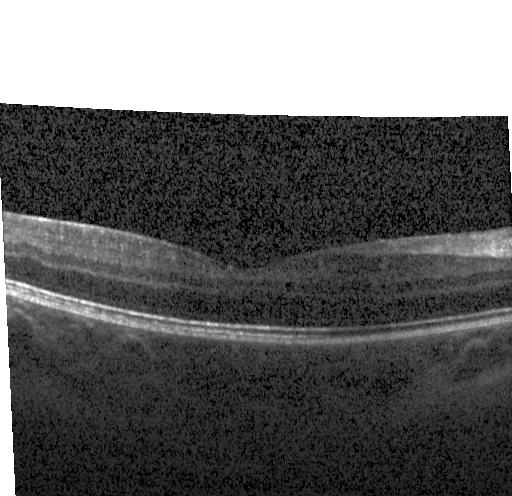 Impression: diabetic macular edema (DME).